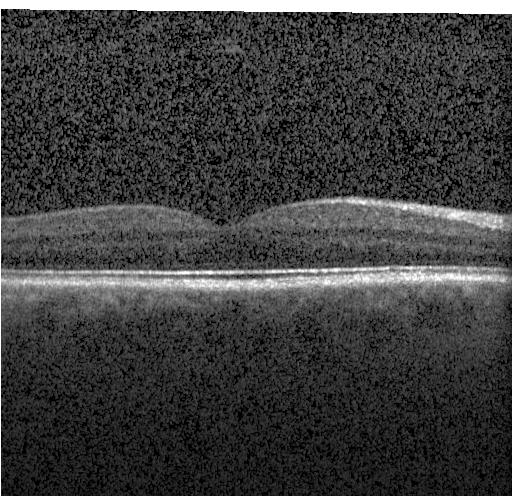 Dx: no choroidal neovascularization, no diabetic macular edema, and no drusen.